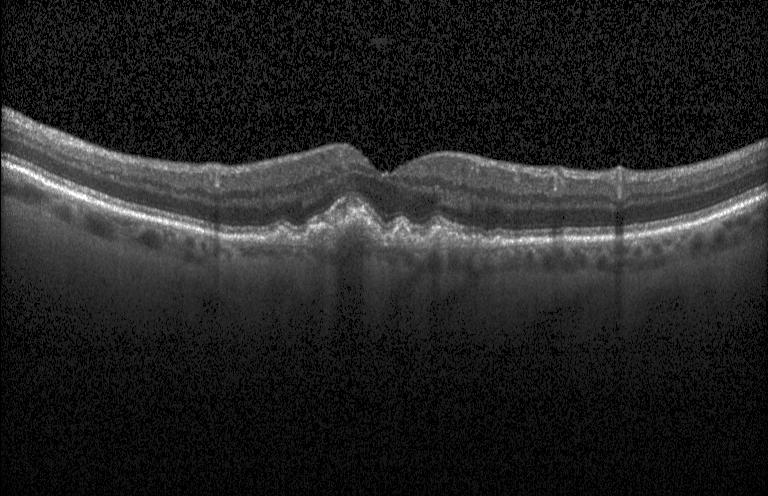 Acquired on a Heidelberg Spectralis · centered on the fovea · retinal OCT cross-section.
The scan shows CNV.